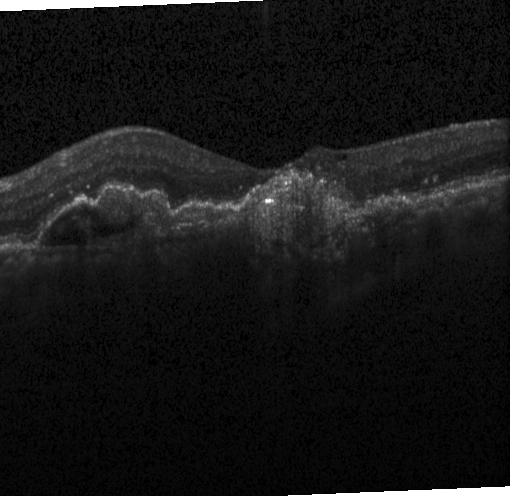

OCT B-scan · spectral-domain optical coherence tomography. Impression: a choroidal neovascular membrane.